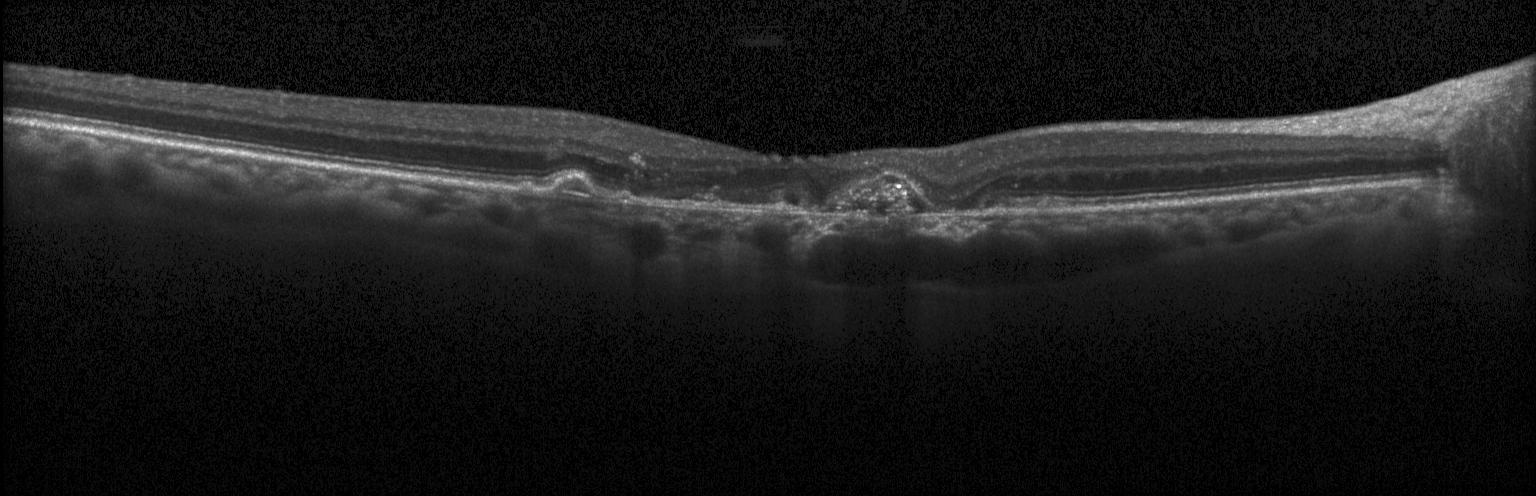

Optical coherence tomography scan. This B-scan demonstrates choroidal neovascularization.